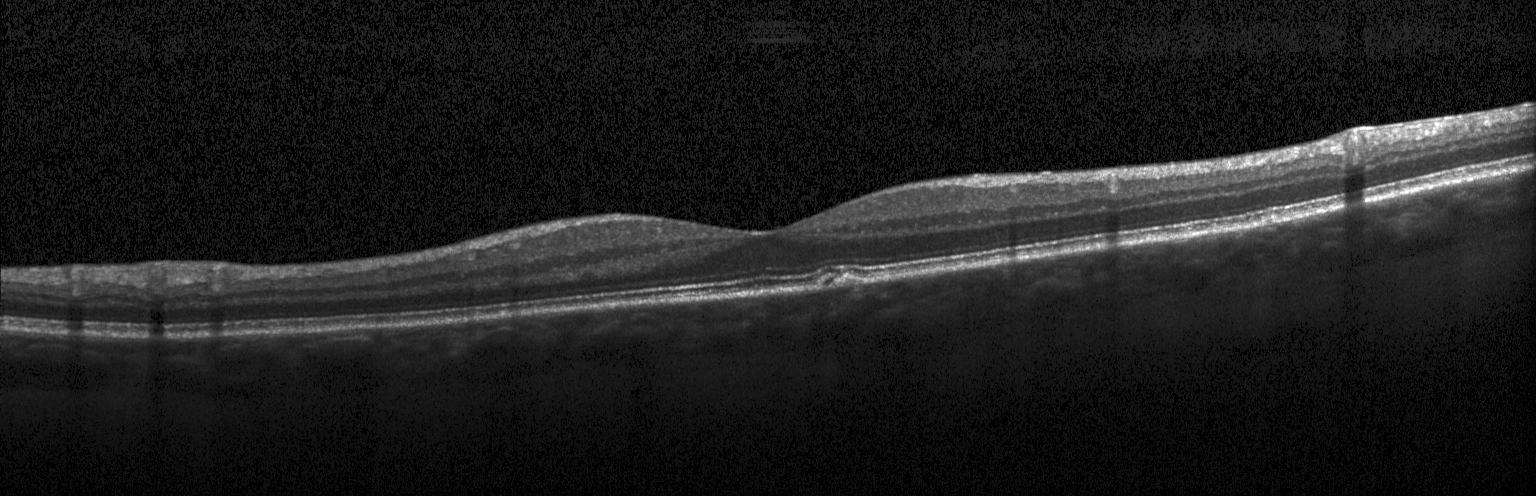
The scan shows multiple drusen.